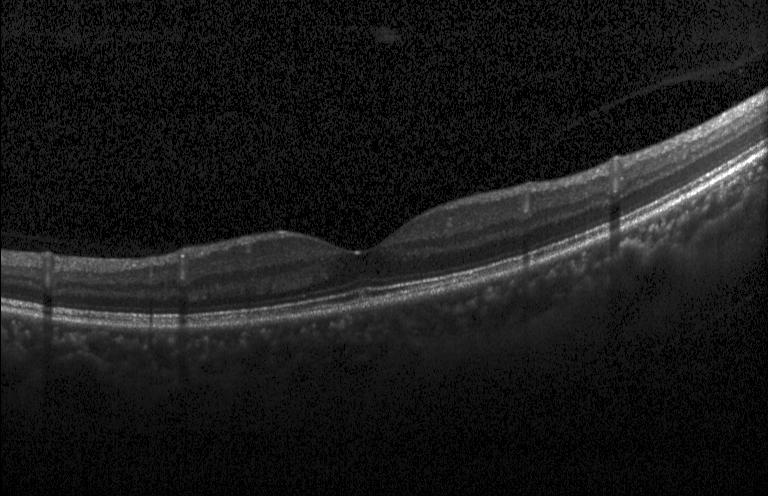
Instrument: Heidelberg Spectralis, OCT line scan. Finding: no choroidal neovascularization, no diabetic macular edema, and no drusen.